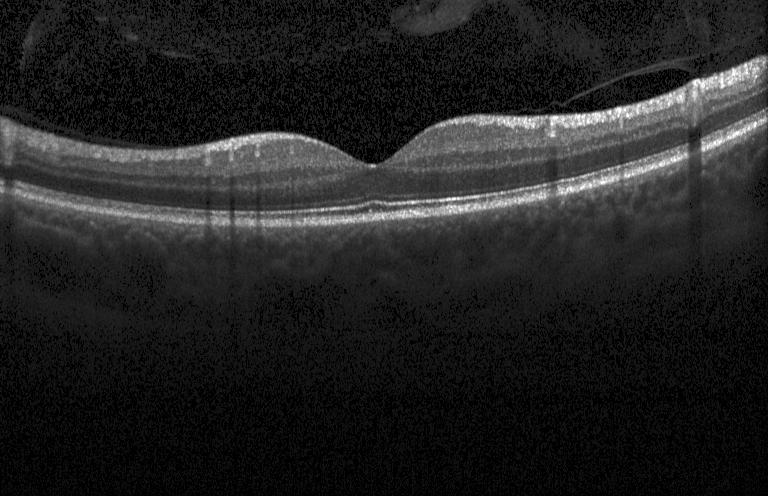 Centered on the fovea, OCT B-scan. Dx: no evidence of choroidal neovascularization, diabetic macular edema, or drusen.